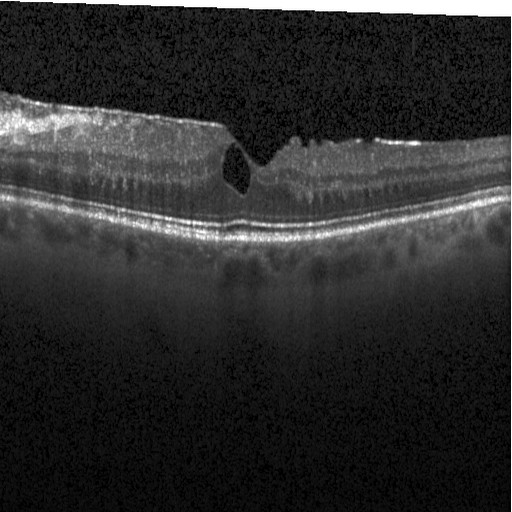

SD-OCT · macular scan · OCT line scan · instrument: Heidelberg Spectralis. Finding: diabetic macular edema (DME).